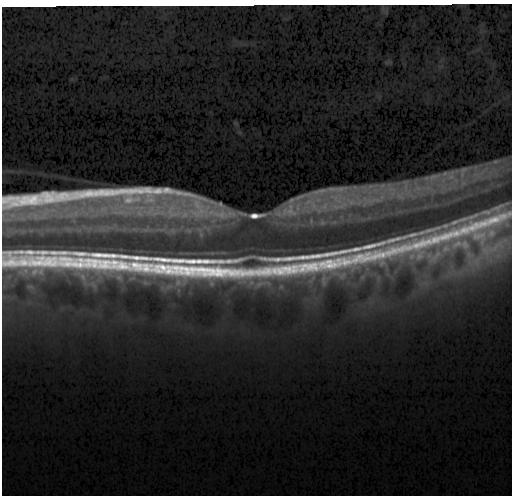 OCT line scan — No evidence of choroidal neovascularization, diabetic macular edema, or drusen.